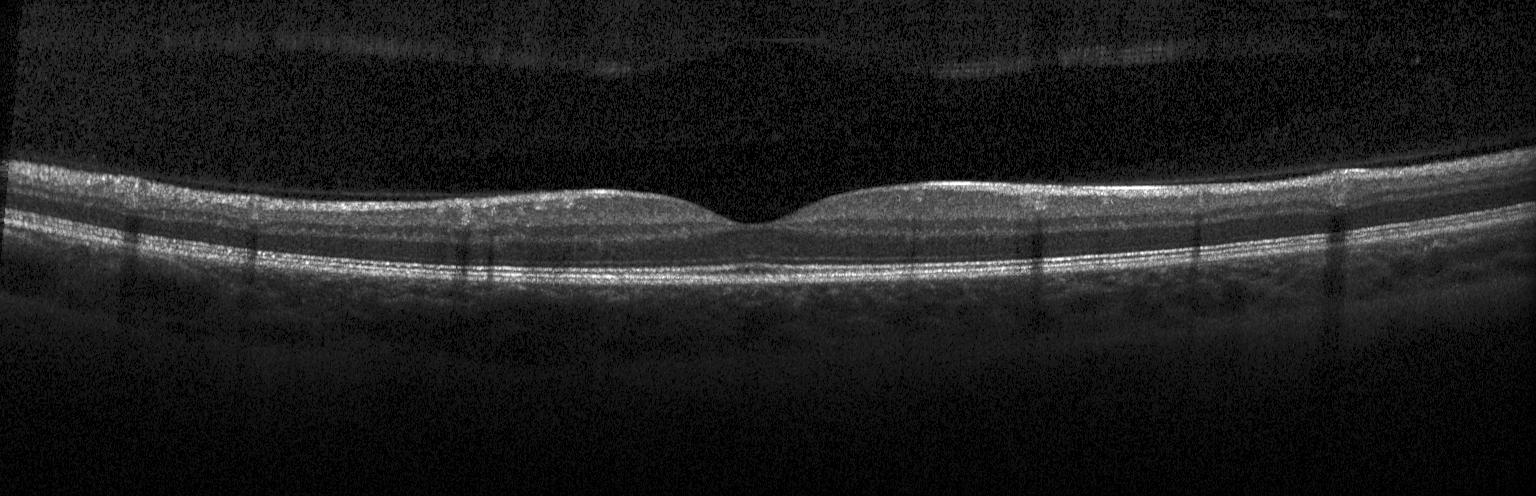
Instrument: Heidelberg Spectralis · retinal OCT B-scan · spectral-domain optical coherence tomography — Impression: no evidence of choroidal neovascularization, diabetic macular edema, or drusen.